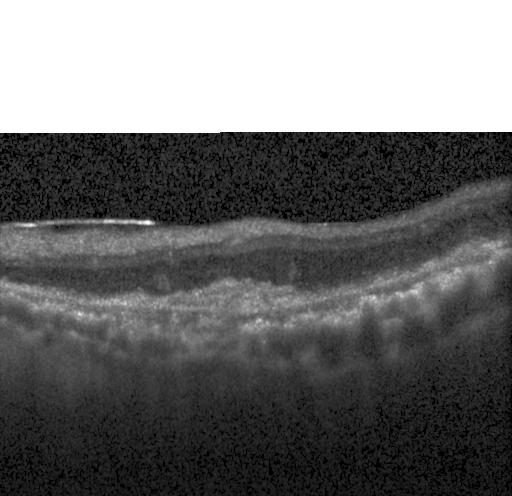
Macular OCT: choroidal neovascularization (CNV).